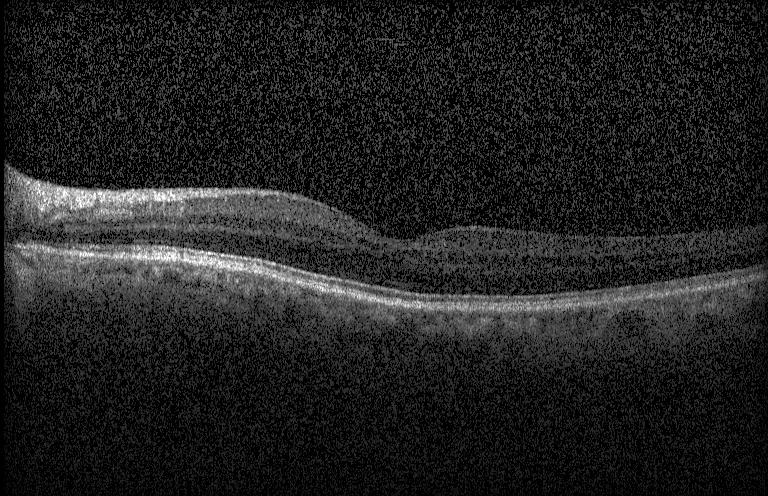
Fovea-centered · optical coherence tomography B-scan — OCT finding: no evidence of choroidal neovascularization, diabetic macular edema, or drusen.